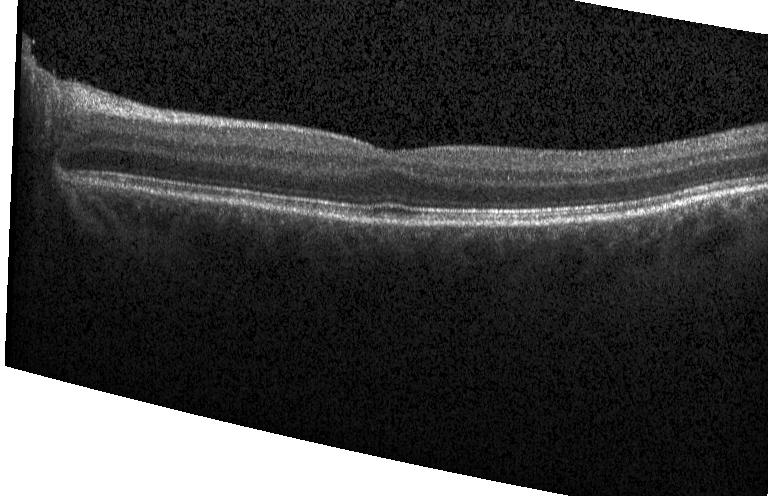

Spectral-domain optical coherence tomography, optical coherence tomography scan, centered on the fovea — Dx: no evidence of CNV, DME, or drusen.